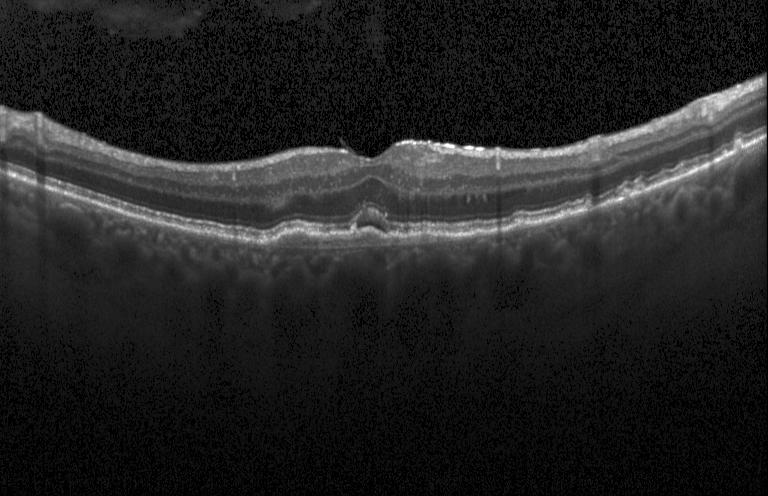
Retinal OCT cross-section, SD-OCT, centered on the fovea, acquired on a Heidelberg Spectralis — Diagnosis: a choroidal neovascular membrane.